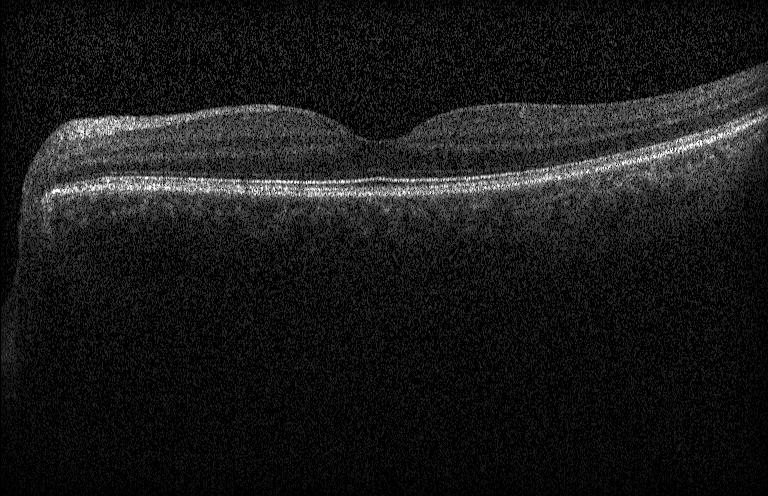
OCT line scan — The scan shows no choroidal neovascularization, diabetic macular edema, or drusen.